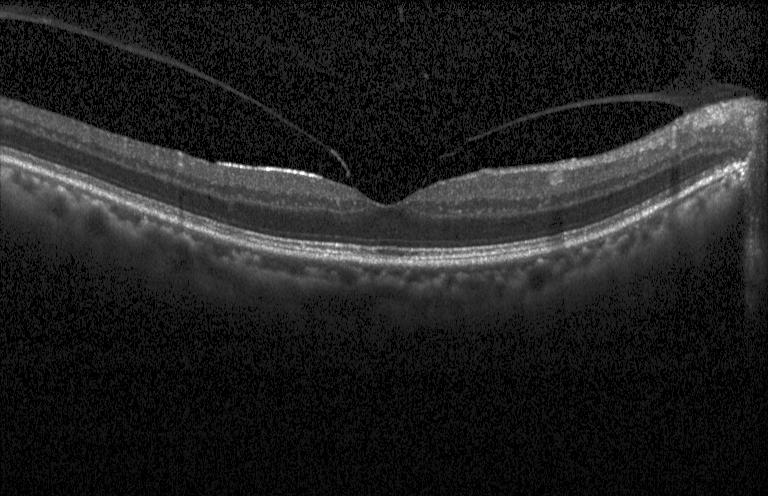 Optical coherence tomography scan — Impression: no choroidal neovascularization, diabetic macular edema, or drusen.